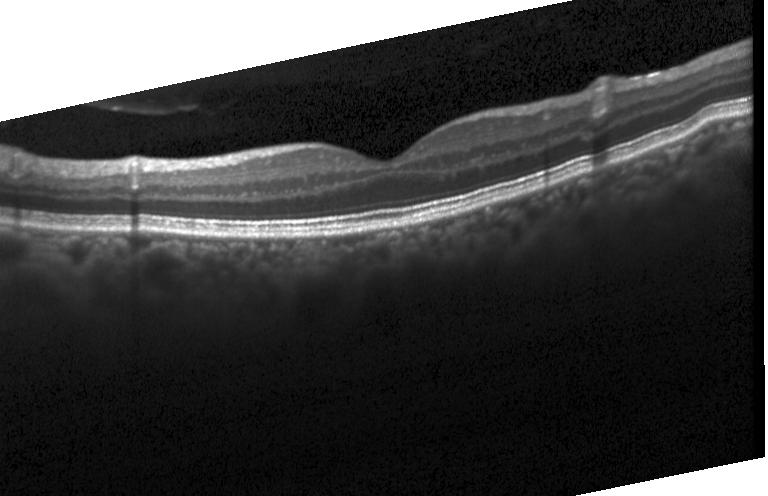
Spectral-domain OCT · retinal OCT cross-section · macular scan · acquired on a Heidelberg Spectralis — Diagnosis: neither choroidal neovascularization, diabetic macular edema, nor drusen.